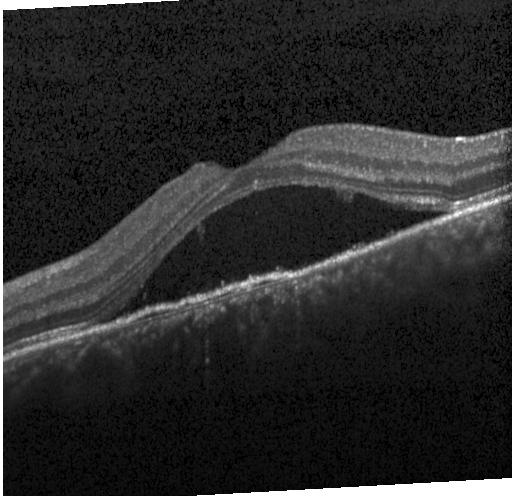 This B-scan demonstrates a choroidal neovascular membrane.